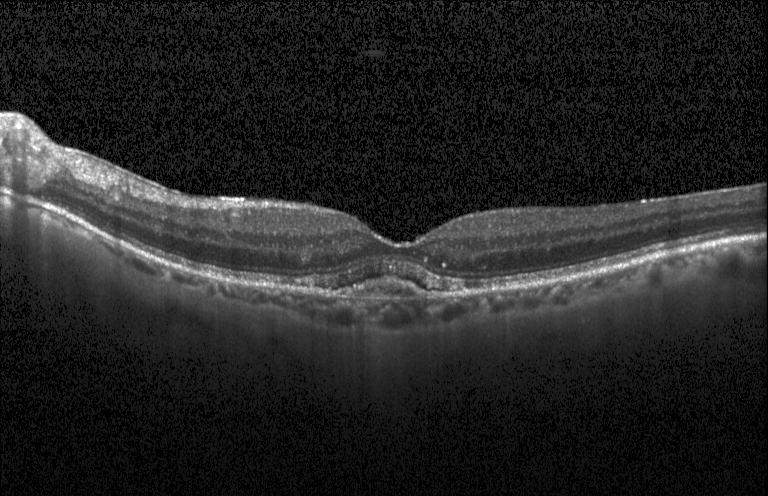 SD-OCT · OCT B-scan — Finding: CNV.